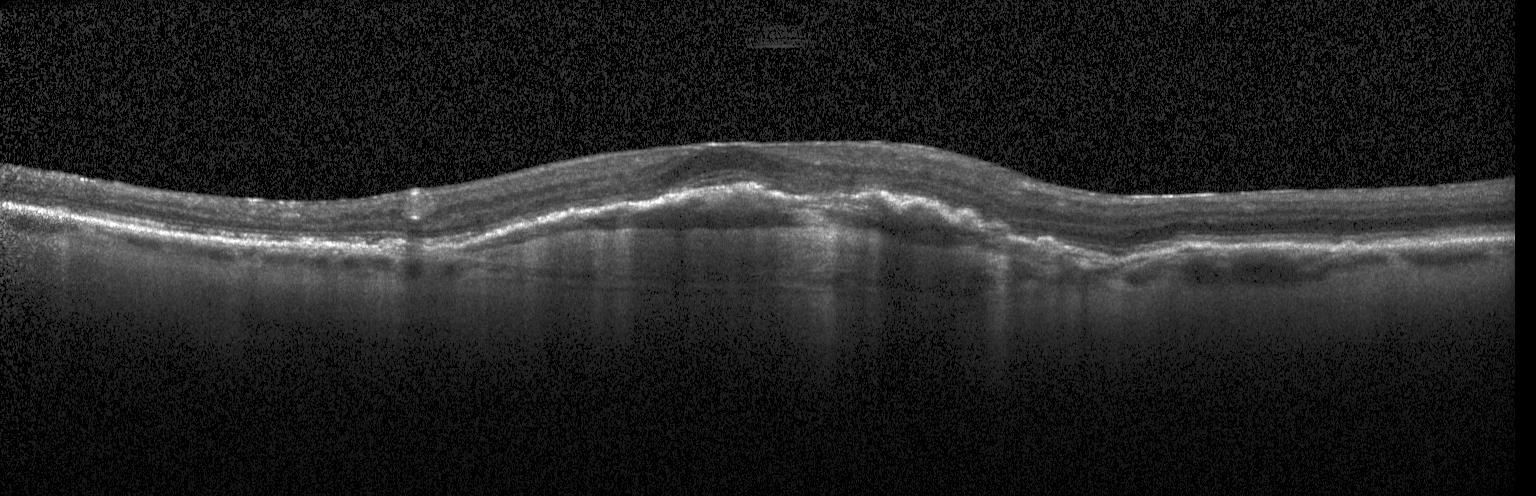 This B-scan demonstrates choroidal neovascularization (CNV).